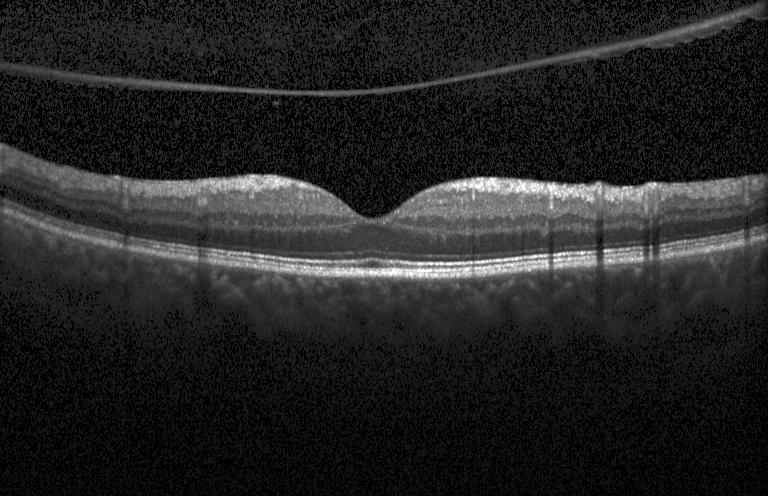 Optical coherence tomography scan — The scan shows neither choroidal neovascularization, diabetic macular edema, nor drusen.